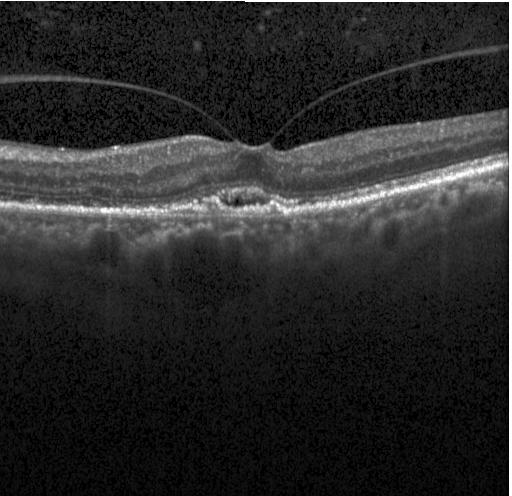 Finding: a choroidal neovascular membrane.